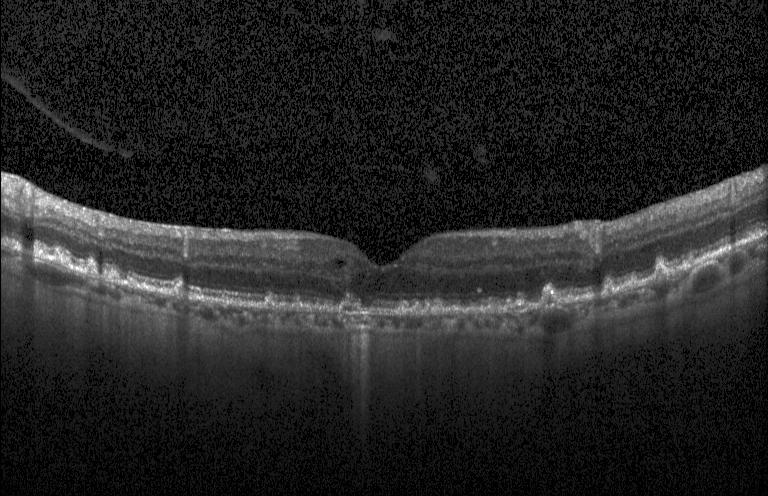
Dx: a choroidal neovascular membrane.